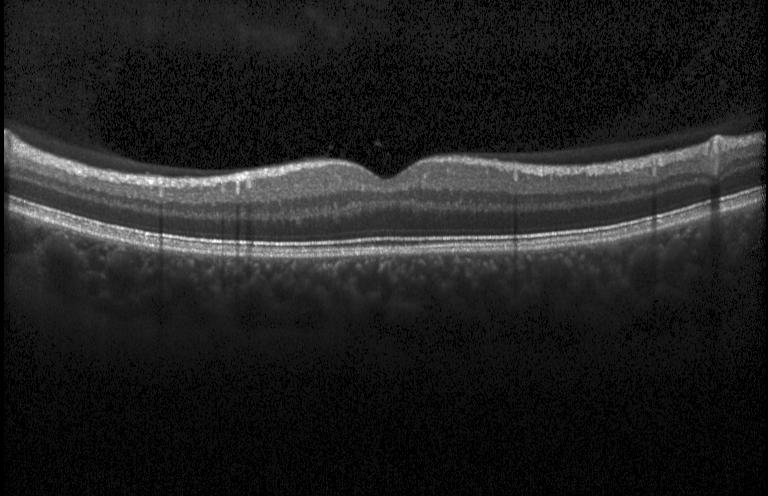
Heidelberg Spectralis OCT system; optical coherence tomography B-scan.
Assessment: no CNV, DME, or drusen.